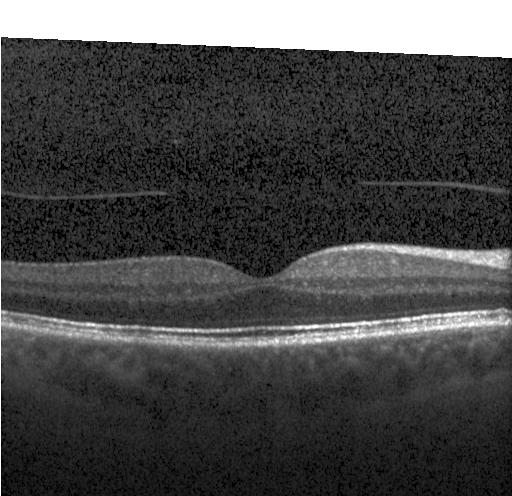 No choroidal neovascularization, diabetic macular edema, or drusen.